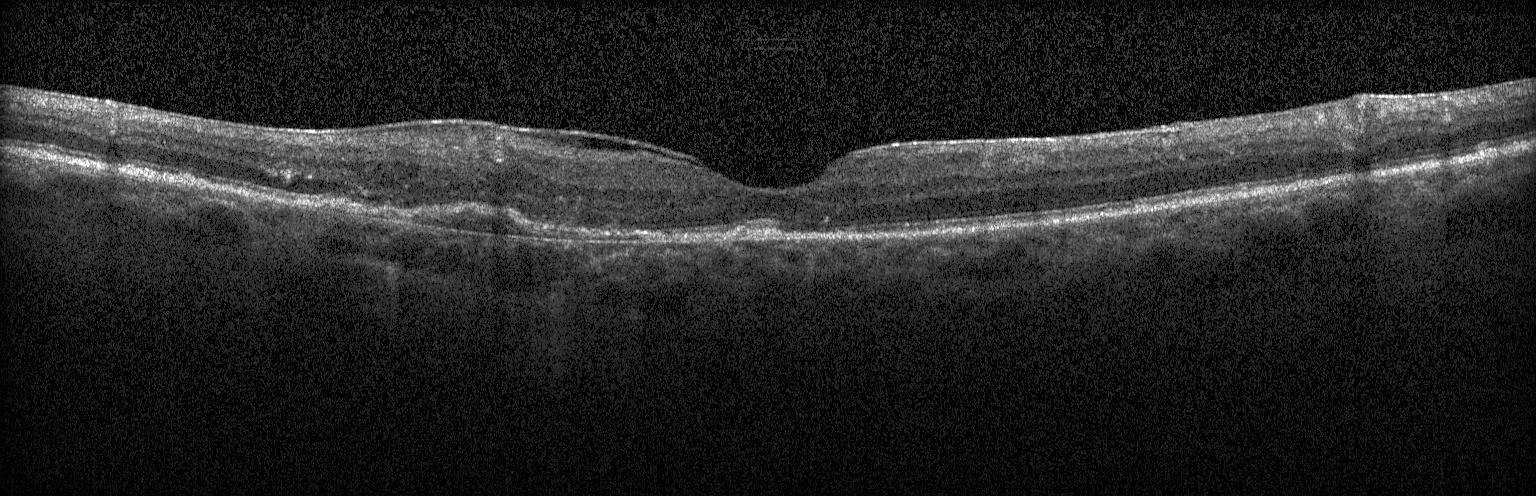 Retinal OCT B-scan
The scan shows choroidal neovascularization (CNV).